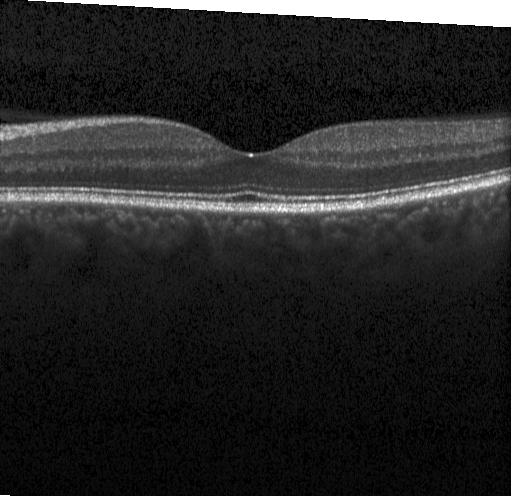 Spectral-domain OCT, OCT line scan, Heidelberg Spectralis.
The scan shows no CNV, no DME, and no drusen.